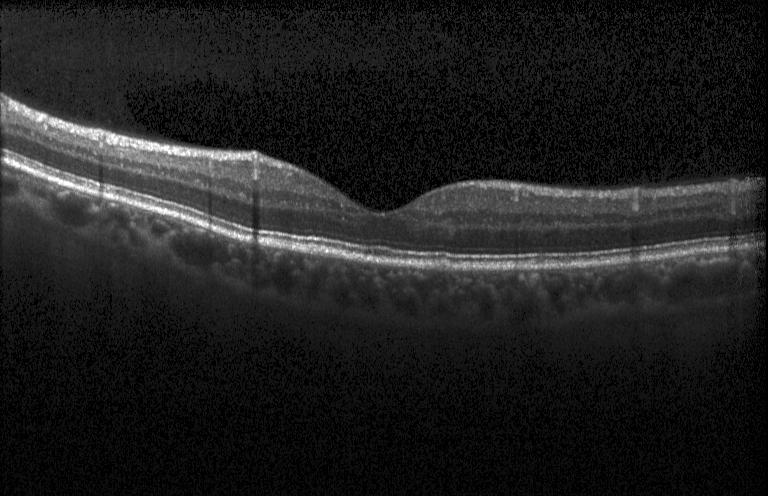
Optical coherence tomography scan
Diagnosis: no choroidal neovascularization, no diabetic macular edema, and no drusen.